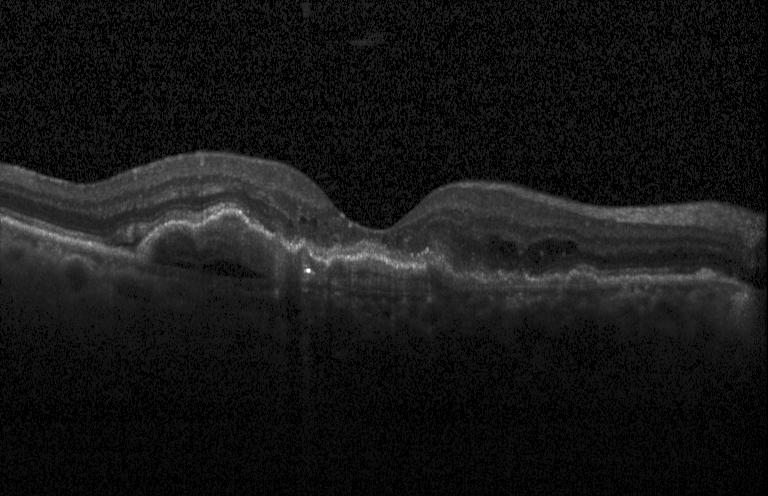
OCT B-scan; Heidelberg Spectralis
Impression: a choroidal neovascular membrane.